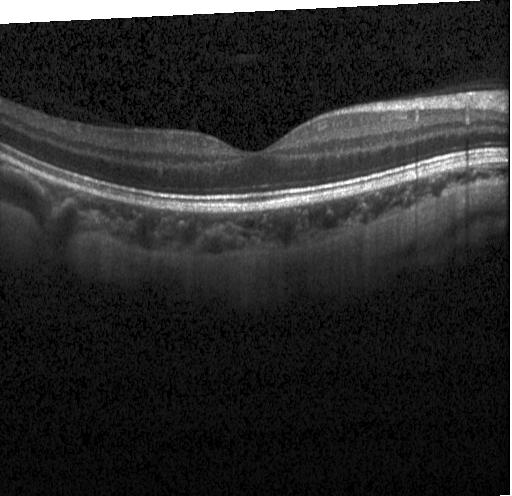 Spectral-domain OCT, OCT B-scan. Finding: neither CNV, DME, nor drusen.